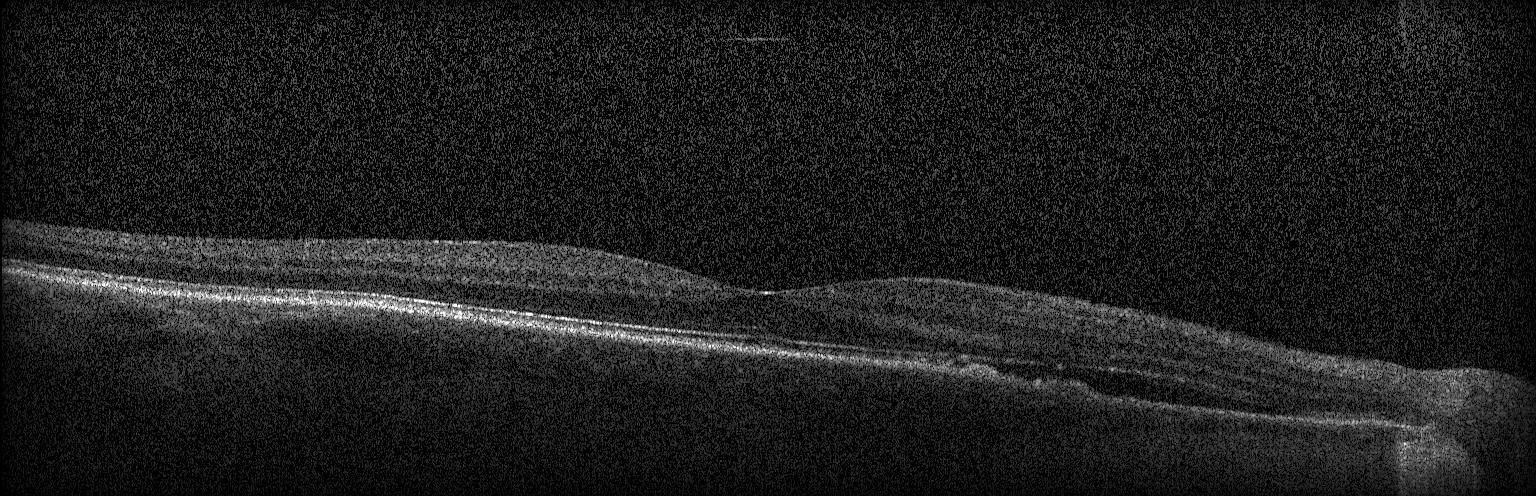 Optical coherence tomography B-scan, fovea-centered, spectral-domain OCT, Heidelberg Spectralis.
Diagnosis: choroidal neovascularization.